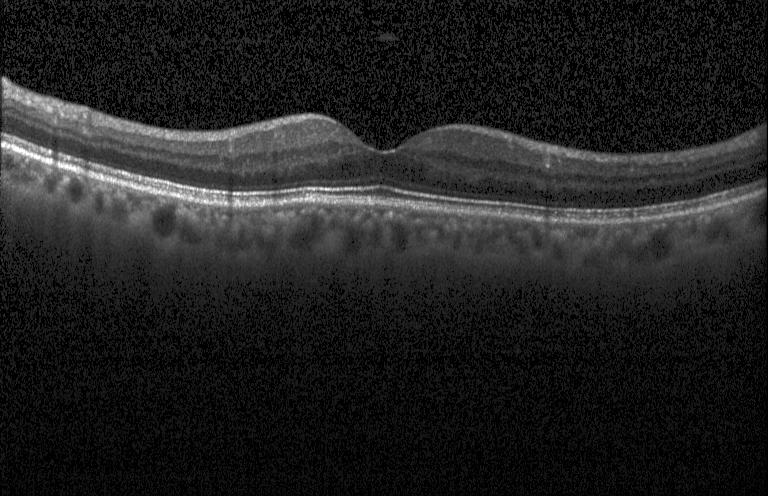

Diagnosis: neither choroidal neovascularization, diabetic macular edema, nor drusen.